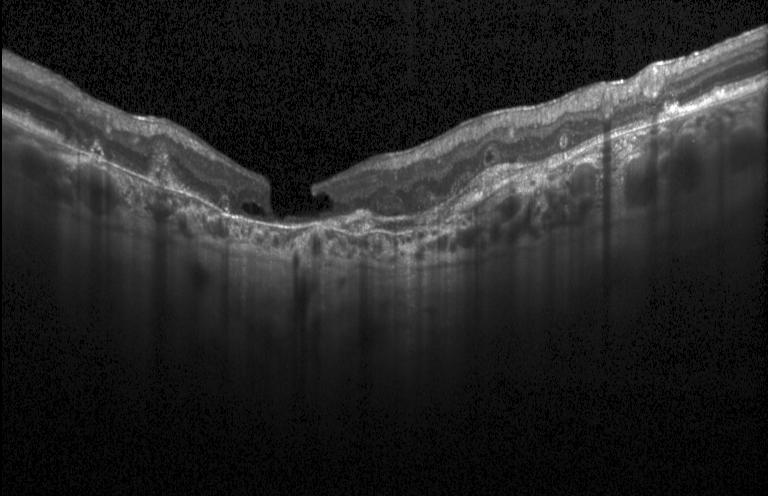
Assessment: a choroidal neovascular membrane.